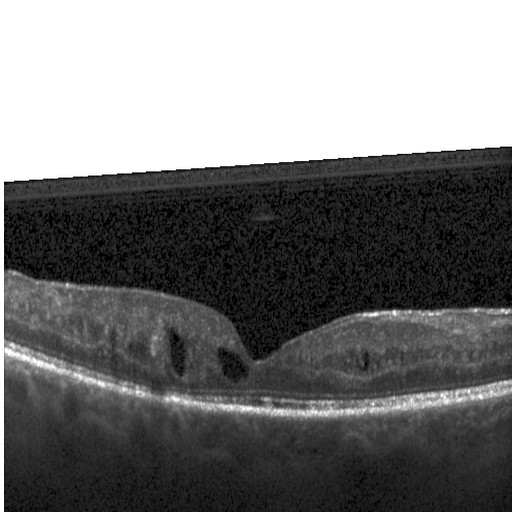 Retinal OCT cross-section, acquired on a Heidelberg Spectralis — This B-scan demonstrates diabetic macular edema.